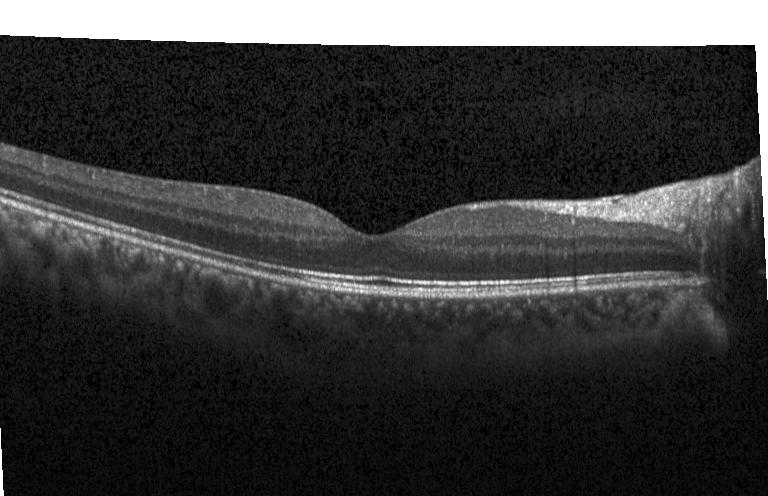
Retinal OCT cross-section showing no choroidal neovascularization, diabetic macular edema, or drusen.